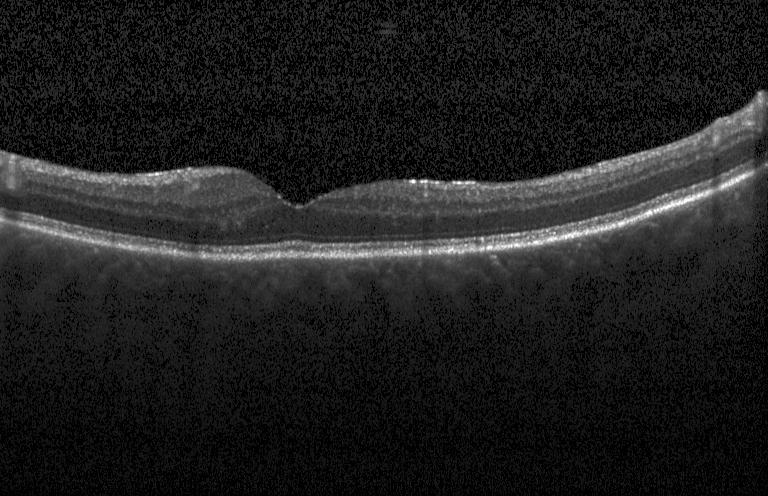 OCT line scan
Diagnosis: no CNV, no DME, and no drusen.